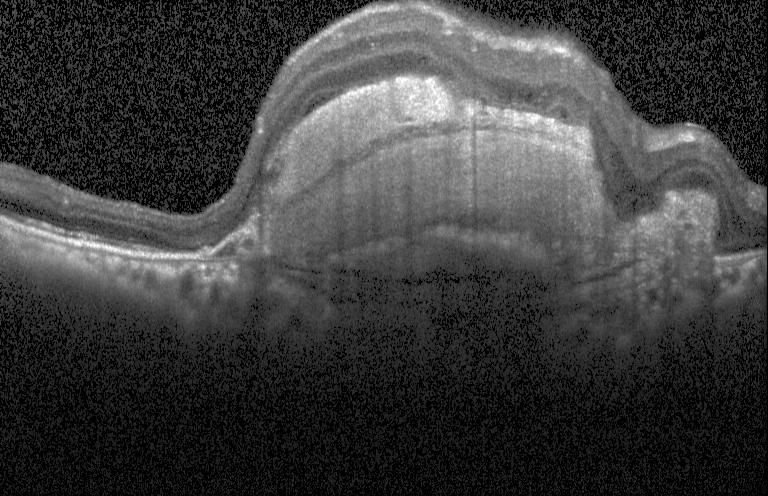
Macular scan; optical coherence tomography scan
Dx: CNV.